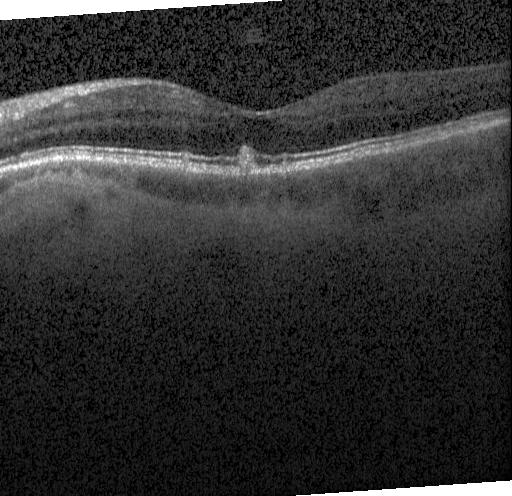
Diagnosis: sub-RPE drusenoid deposits.